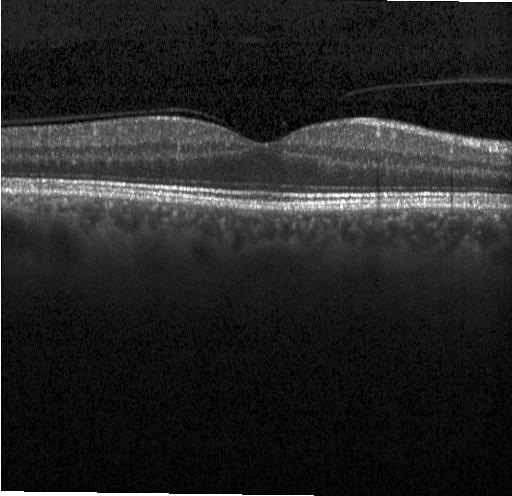
Acquired on a Heidelberg Spectralis · OCT B-scan
Assessment: no evidence of CNV, DME, or drusen.